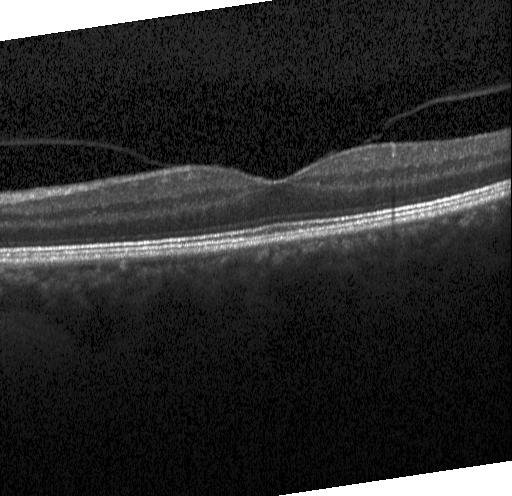

Horizontal scan through the fovea · optical coherence tomography scan.
Dx: no choroidal neovascularization, no diabetic macular edema, and no drusen.